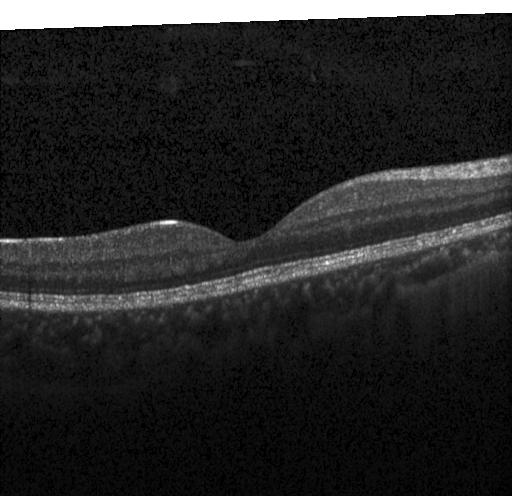 Macular OCT demonstrating no evidence of choroidal neovascularization, diabetic macular edema, or drusen.